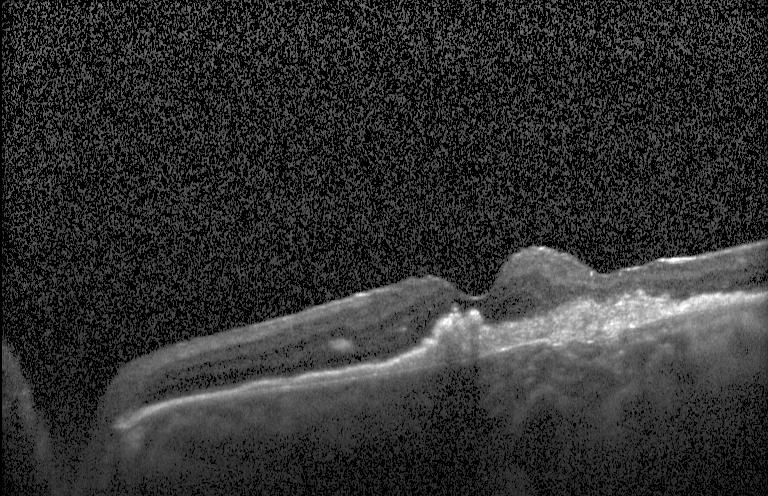

OCT line scan — Finding: choroidal neovascularization.